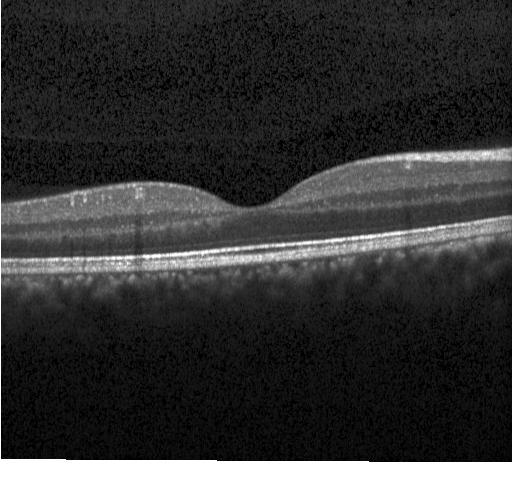
Optical coherence tomography scan. Heidelberg Spectralis. Spectral-domain optical coherence tomography
Impression: no evidence of choroidal neovascularization, diabetic macular edema, or drusen.